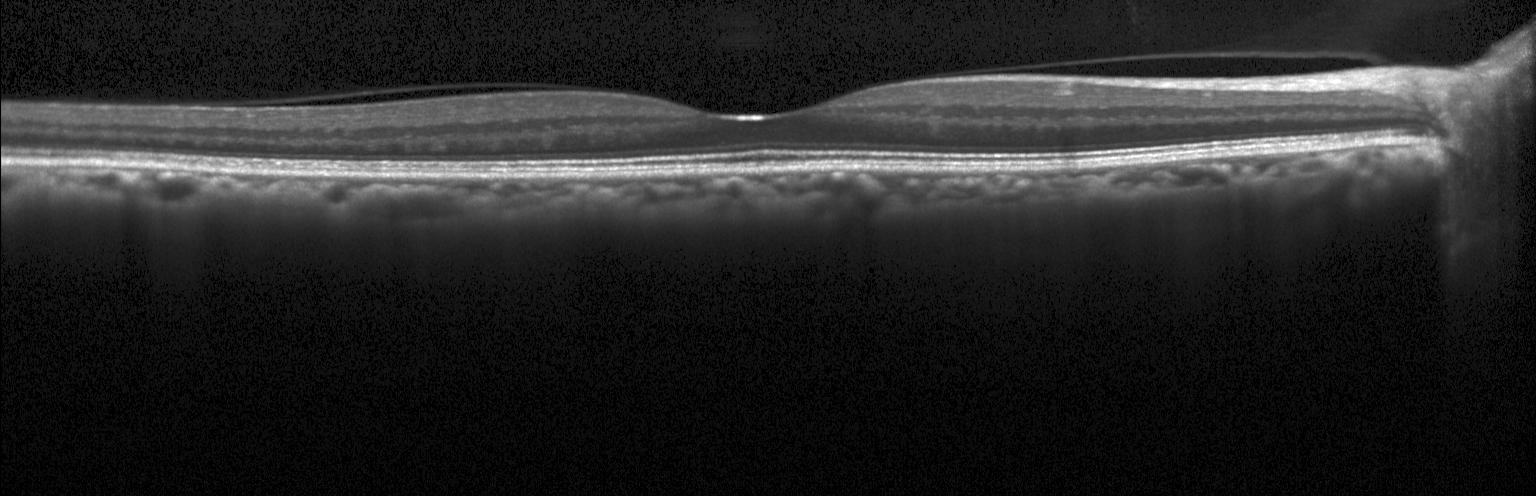

The scan shows neither choroidal neovascularization, diabetic macular edema, nor drusen.